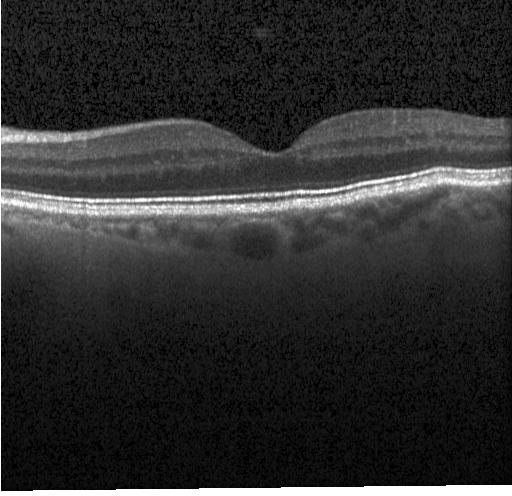
The scan shows neither choroidal neovascularization, diabetic macular edema, nor drusen.